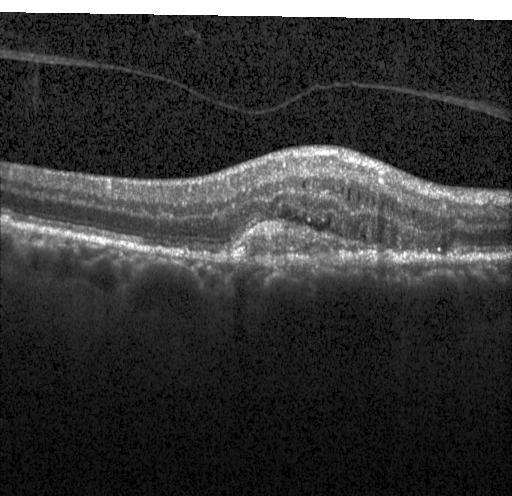

Optical coherence tomography B-scan
The scan shows a choroidal neovascular membrane.